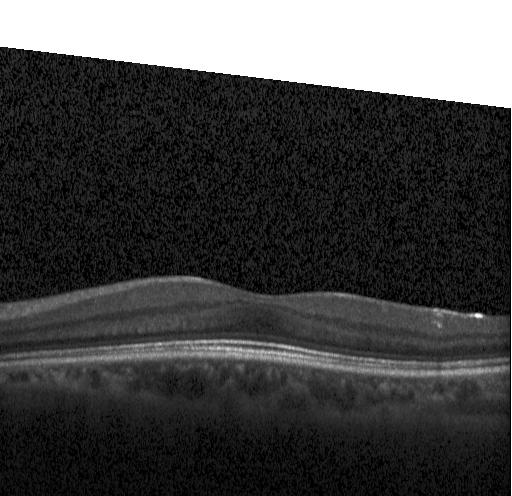
OCT B-scan showing no choroidal neovascularization, no diabetic macular edema, and no drusen.